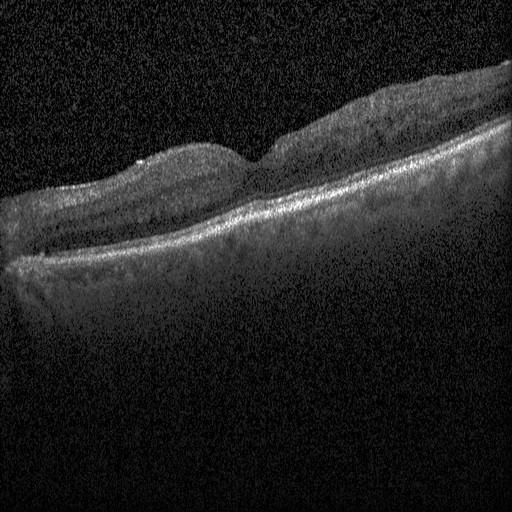
OCT line scan. Centered on the fovea — Dx: diabetic macular edema (DME).